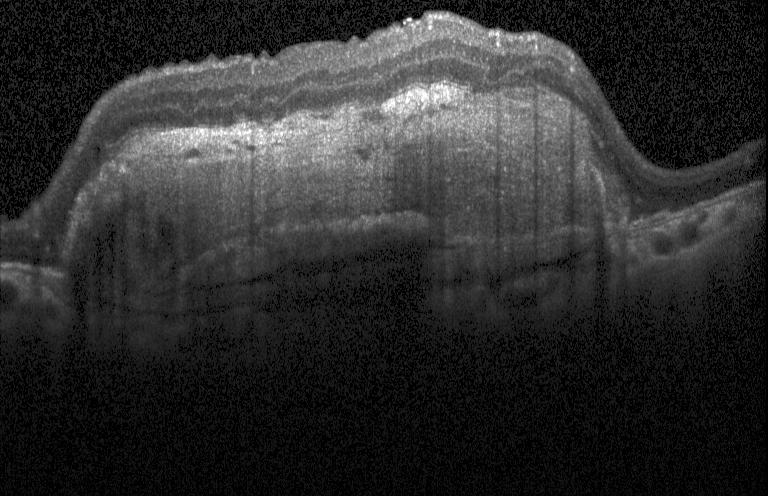
OCT B-scan, macular scan, spectral-domain optical coherence tomography, instrument: Heidelberg Spectralis.
Diagnosis: a choroidal neovascular membrane.